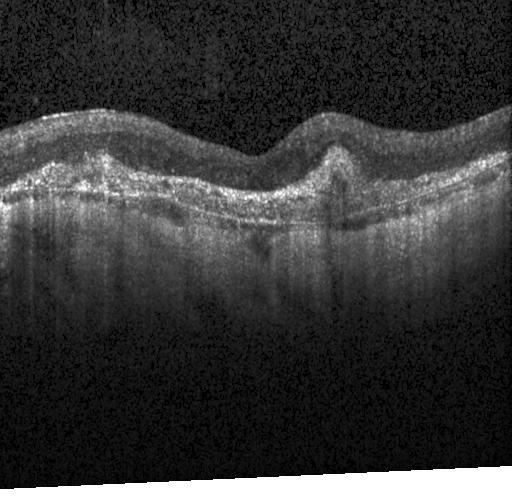
Diagnosis: a choroidal neovascular membrane.